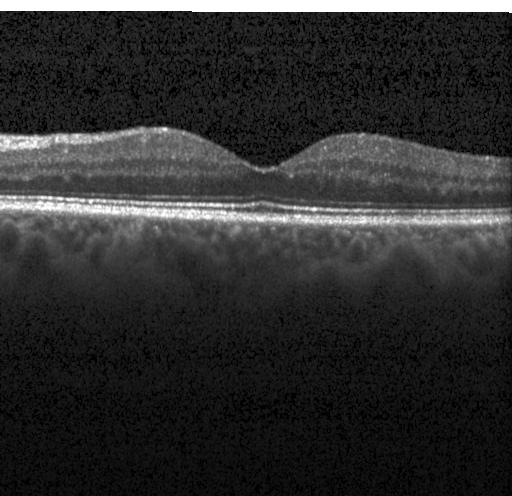 Retinal OCT B-scan — Diagnosis: neither choroidal neovascularization, diabetic macular edema, nor drusen.